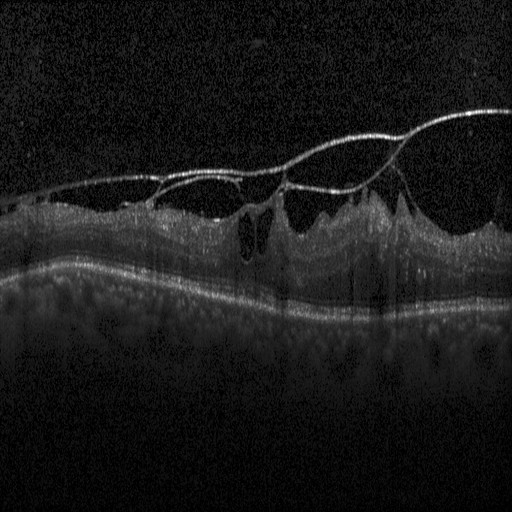
Optical coherence tomography scan. This B-scan demonstrates diabetic macular edema (DME).